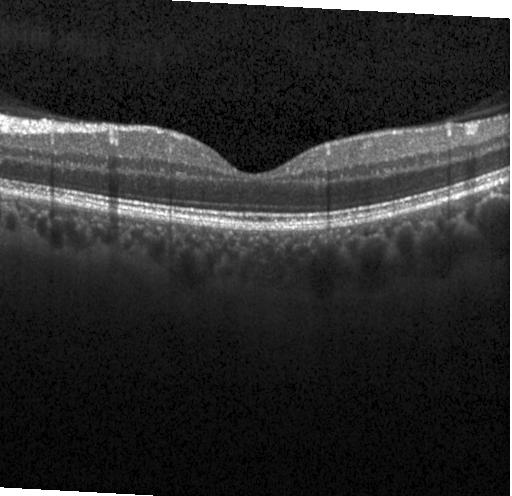 Retinal OCT cross-section showing neither CNV, DME, nor drusen.